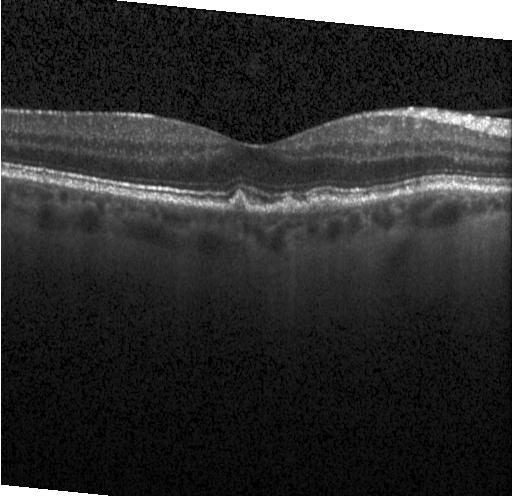

Optical coherence tomography scan.
Assessment: drusen.